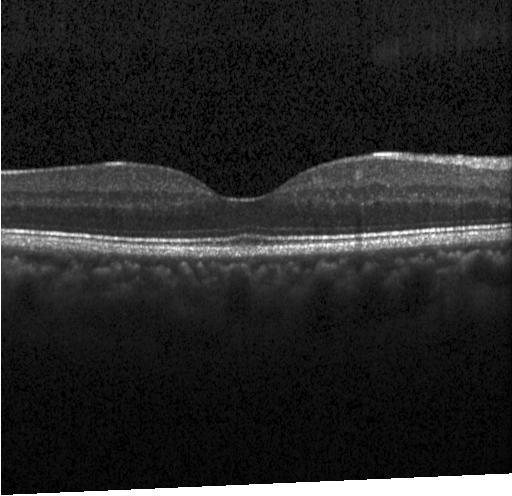
This B-scan demonstrates no evidence of choroidal neovascularization, diabetic macular edema, or drusen.